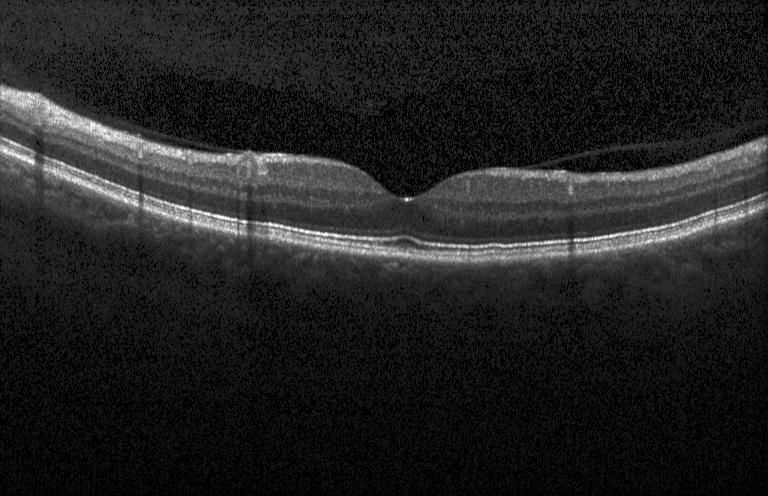 Spectral-domain OCT B-scan: neither choroidal neovascularization, diabetic macular edema, nor drusen.